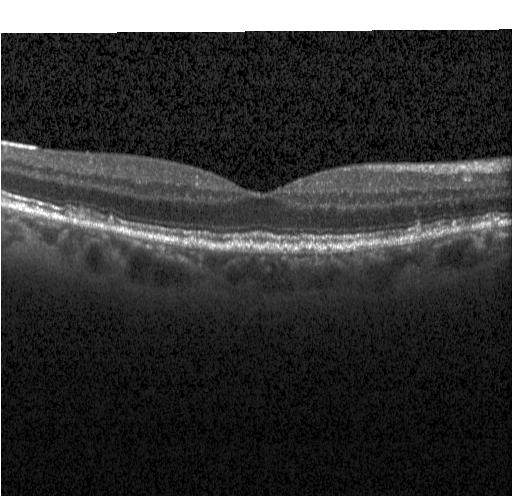
Heidelberg Spectralis · horizontal scan through the fovea · OCT B-scan — Drusen.